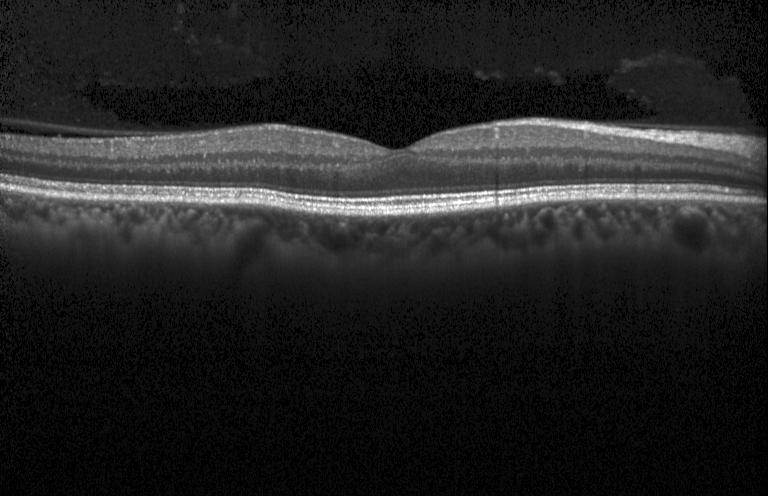

Spectral-domain OCT; OCT line scan.
Impression: neither CNV, DME, nor drusen.